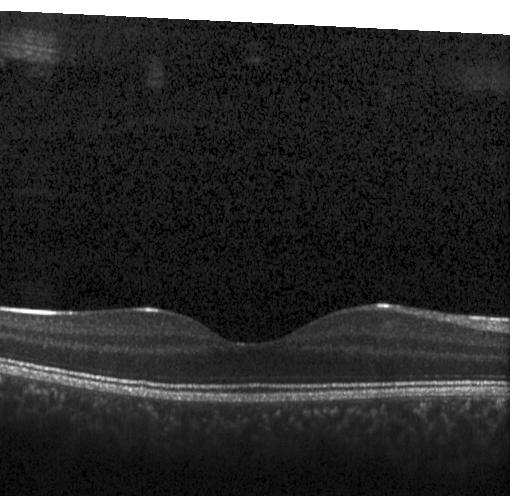 Optical coherence tomography scan
Finding: no choroidal neovascularization, diabetic macular edema, or drusen.